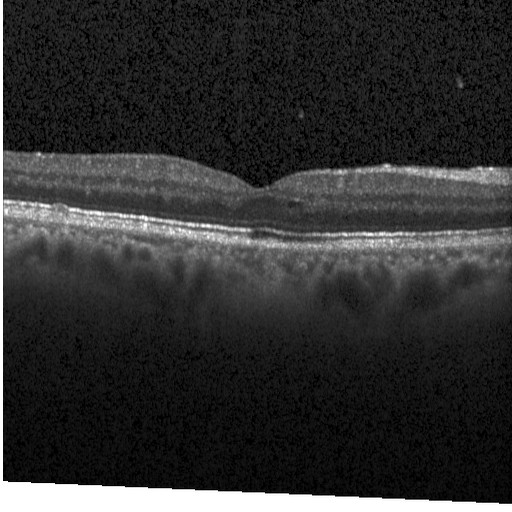
OCT B-scan; SD-OCT
This B-scan demonstrates diabetic macular edema (DME).